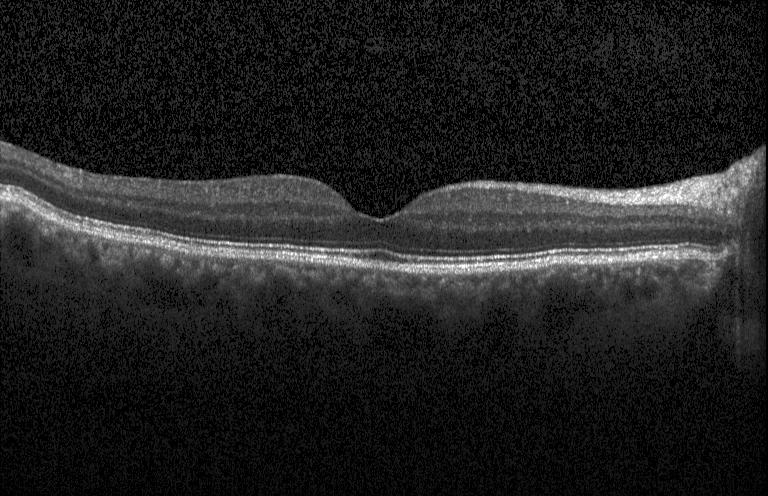

Optical coherence tomography scan.
Diagnosis: neither CNV, DME, nor drusen.